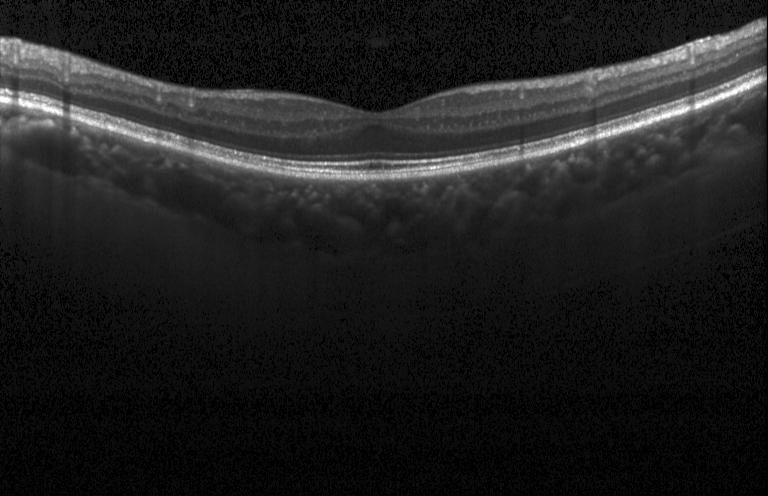

Instrument: Heidelberg Spectralis. SD-OCT. Retinal OCT cross-section
Impression: neither CNV, DME, nor drusen.